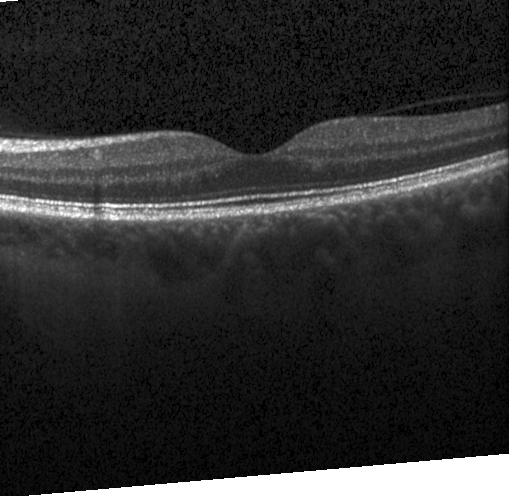
The scan shows no CNV, DME, or drusen.